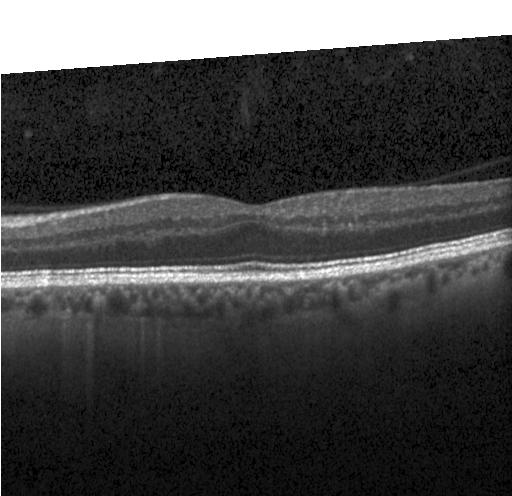

No choroidal neovascularization, no diabetic macular edema, and no drusen.